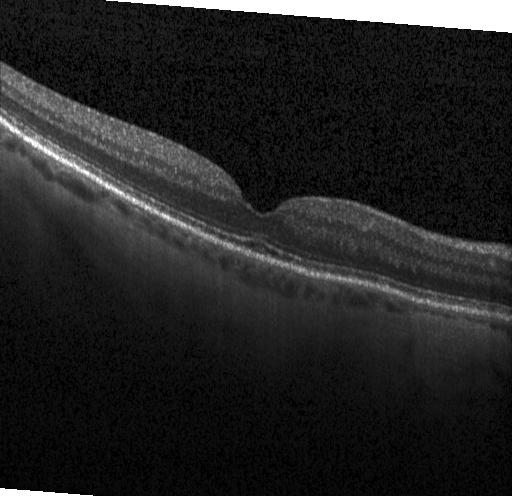 Dx: no evidence of CNV, DME, or drusen.